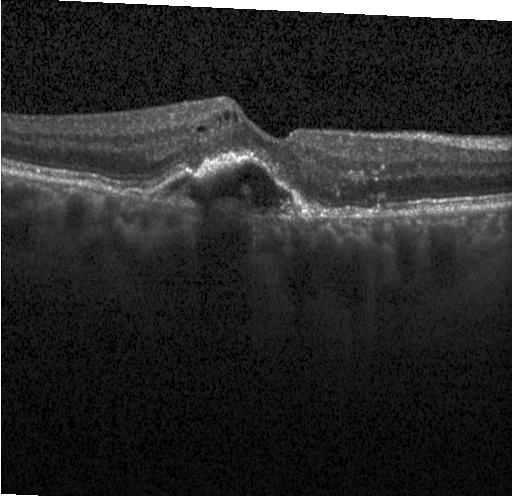
Impression: a choroidal neovascular membrane.